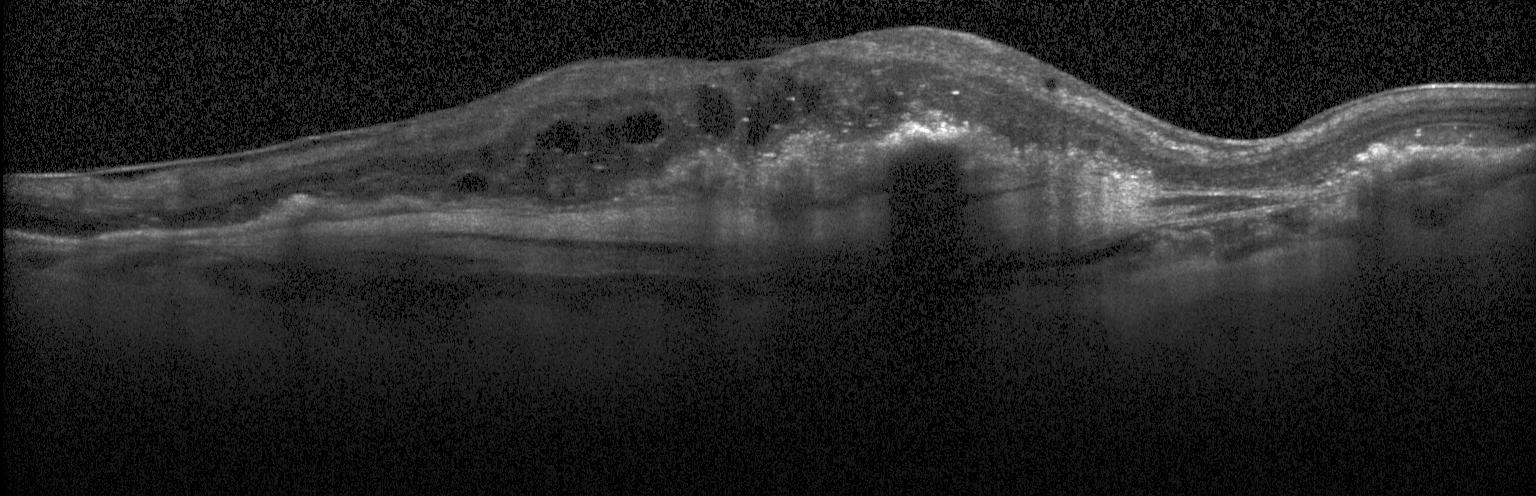
Impression: a choroidal neovascular membrane.